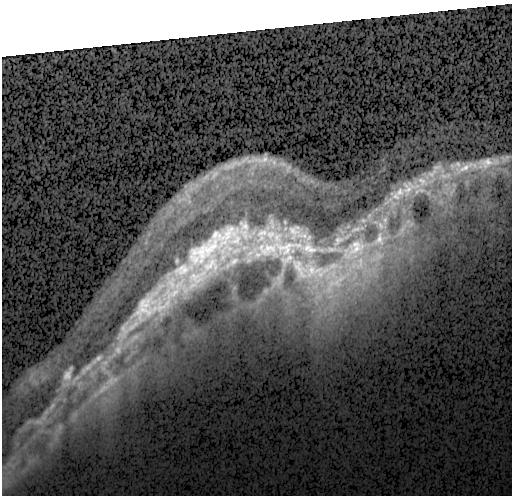
Impression: choroidal neovascularization.